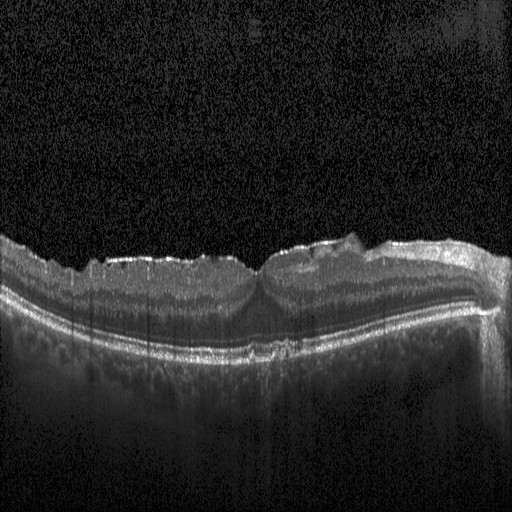

Dx: DME.